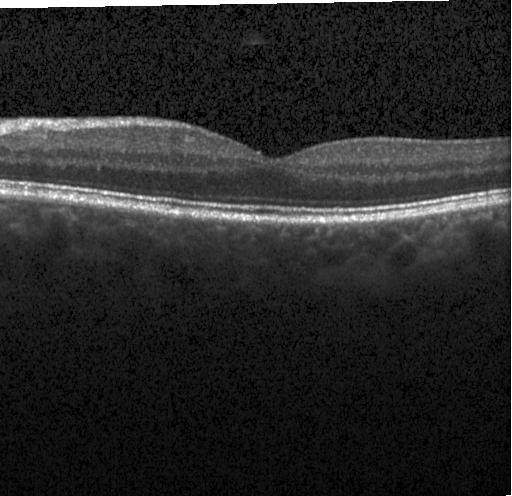
Spectral-domain optical coherence tomography. Retinal OCT B-scan. Fovea-centered. Heidelberg Spectralis OCT system
Assessment: neither CNV, DME, nor drusen.